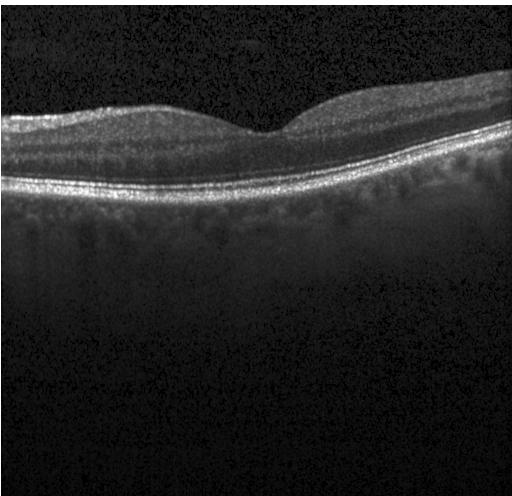
OCT line scan · spectral-domain optical coherence tomography · centered on the fovea · acquired on a Heidelberg Spectralis
Diagnosis: no CNV, no DME, and no drusen.